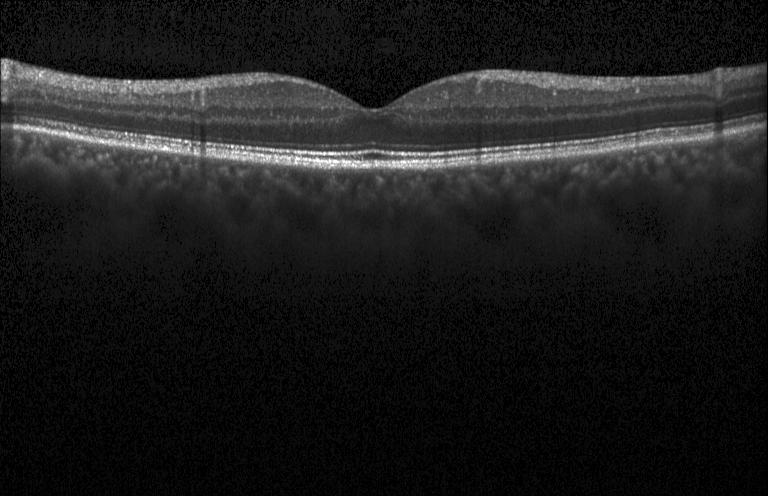
Finding: no evidence of choroidal neovascularization, diabetic macular edema, or drusen.